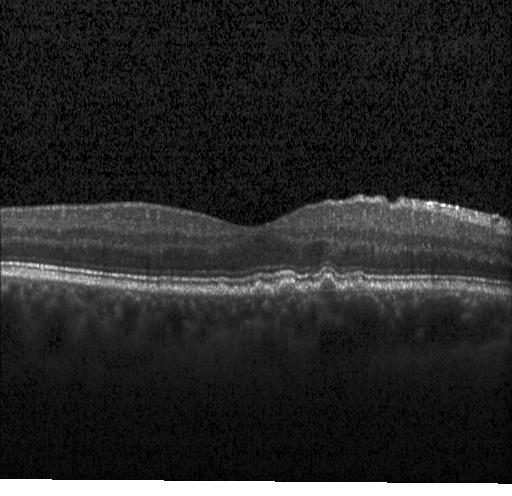
SD-OCT; retinal OCT cross-section; Heidelberg Spectralis OCT system; fovea-centered
Impression: multiple drusen.